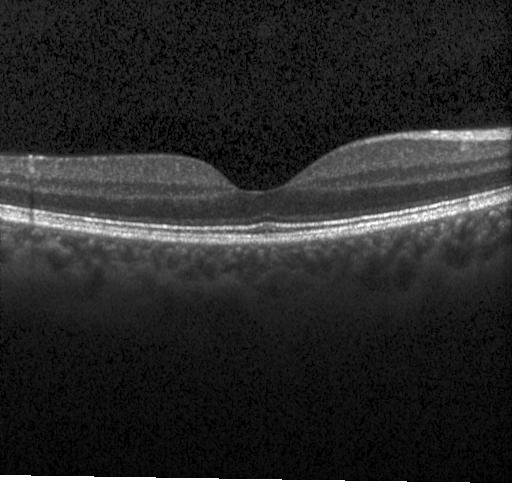

Horizontal scan through the fovea. Acquired on a Heidelberg Spectralis. OCT line scan. SD-OCT — Diagnosis: no choroidal neovascularization, no diabetic macular edema, and no drusen.